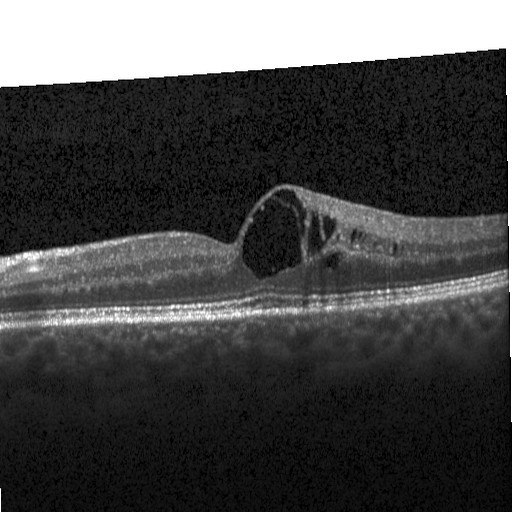

Assessment: diabetic macular edema.